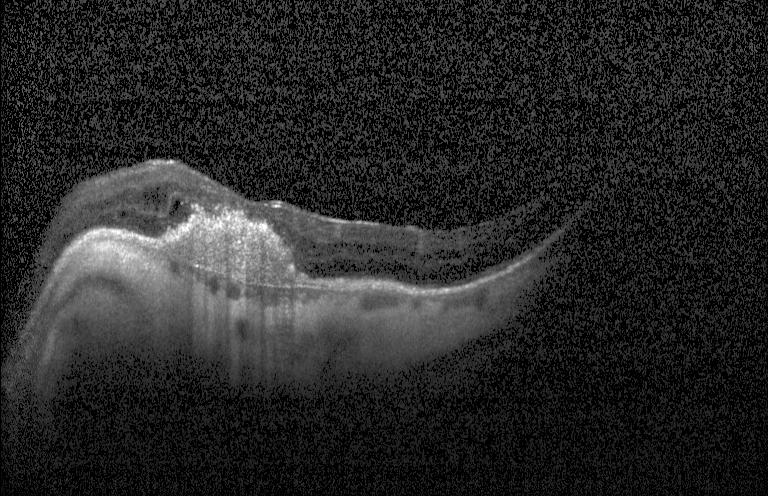

Fovea-centered; spectral-domain OCT; retinal OCT cross-section.
Dx: a choroidal neovascular membrane.